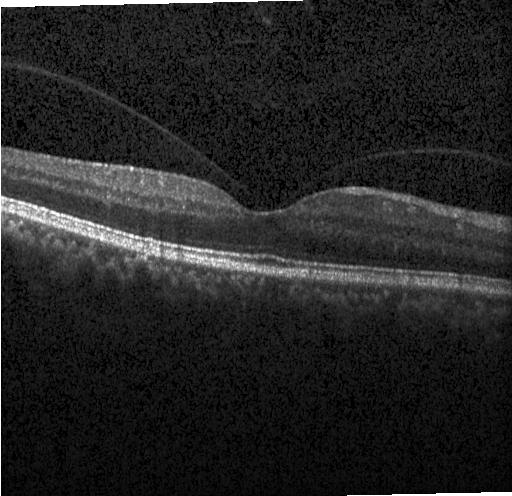

Retinal OCT cross-section; through the macula. Dx: neither CNV, DME, nor drusen.